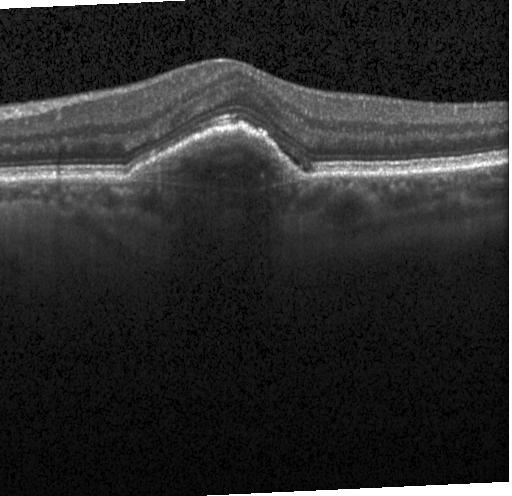 Optical coherence tomography scan, Heidelberg Spectralis, horizontal scan through the fovea, spectral-domain OCT
Finding: CNV.